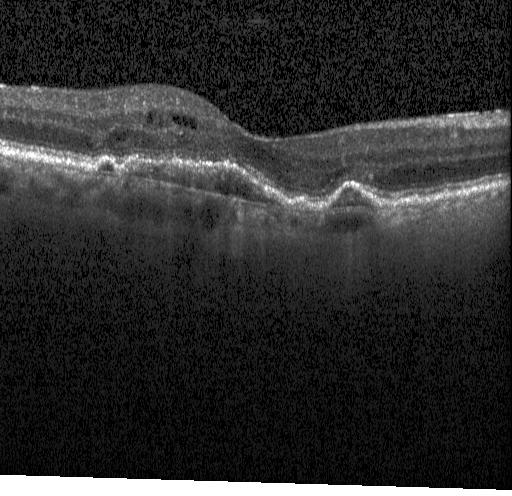 Spectral-domain OCT; horizontal scan through the fovea; retinal OCT B-scan
Impression: a choroidal neovascular membrane.